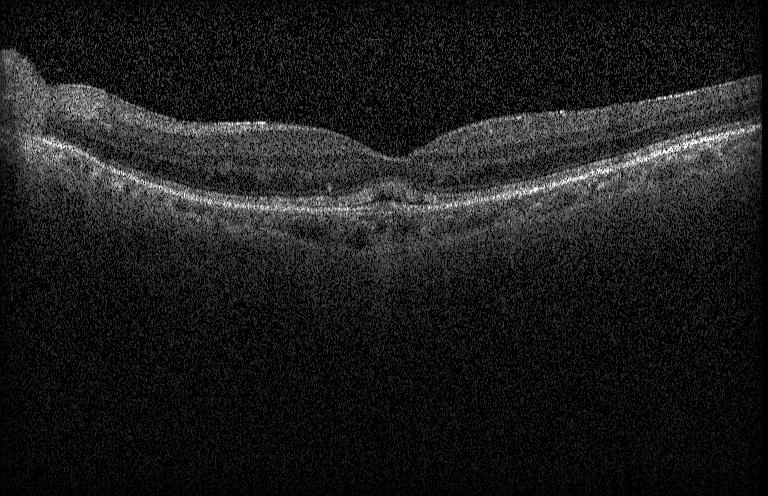 Optical coherence tomography scan — A choroidal neovascular membrane.